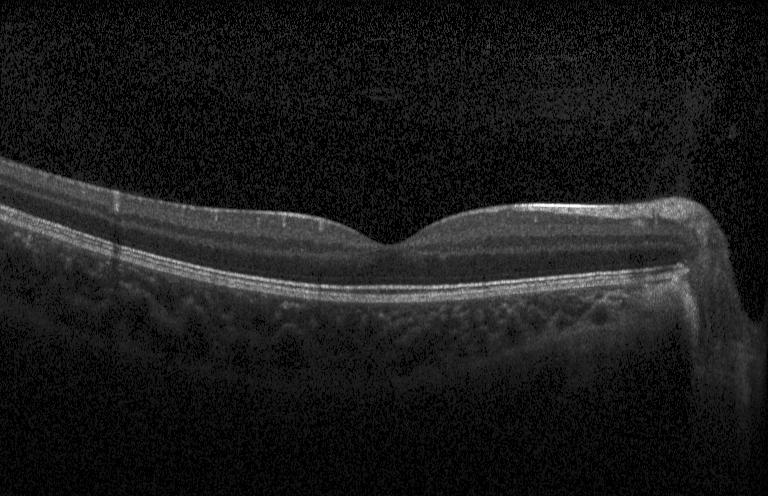
Impression: no evidence of choroidal neovascularization, diabetic macular edema, or drusen.